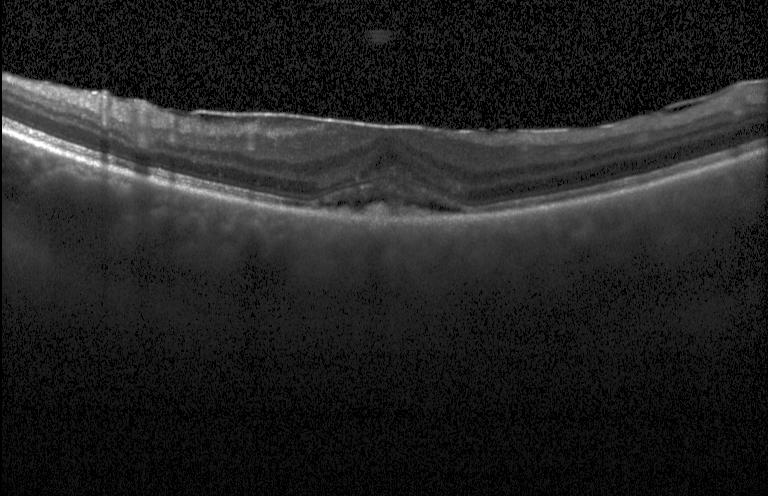
CNV.